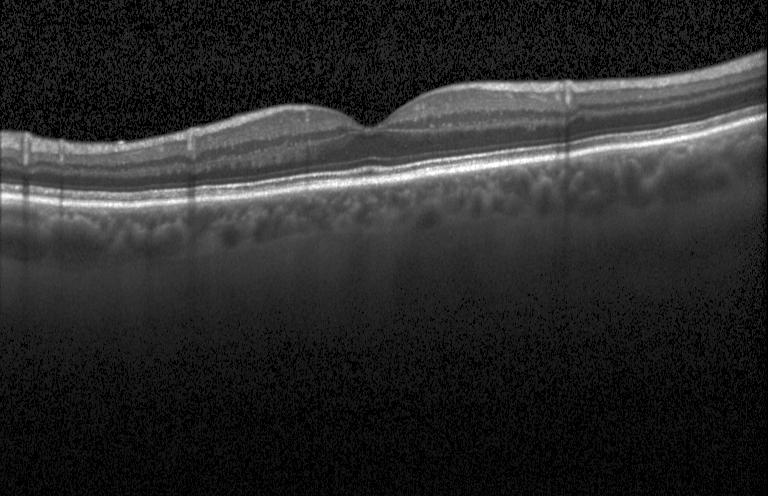 Optical coherence tomography scan. Diagnosis: no choroidal neovascularization, no diabetic macular edema, and no drusen.